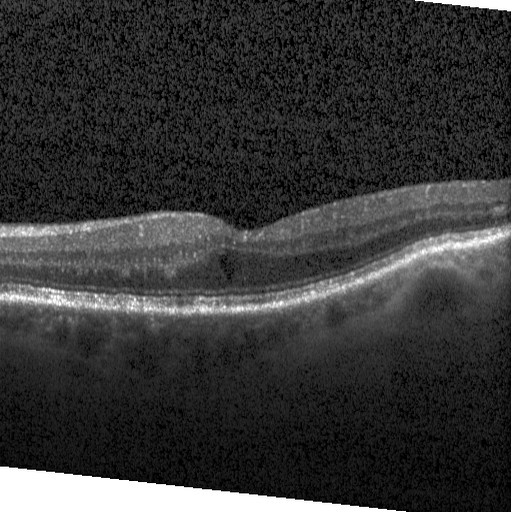 The scan shows diabetic macular edema.